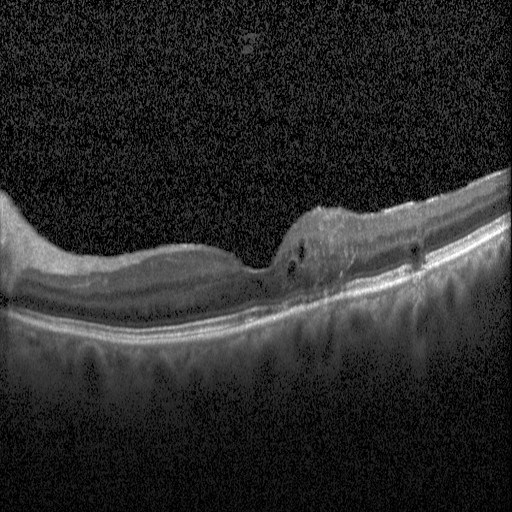
Acquired on a Heidelberg Spectralis, through the macula, OCT B-scan — Assessment: diabetic macular edema.